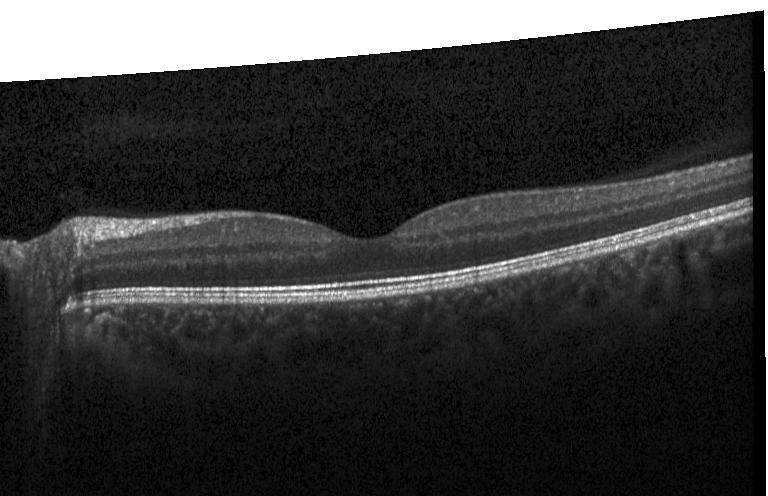 Fovea-centered, optical coherence tomography scan
Finding: no evidence of choroidal neovascularization, diabetic macular edema, or drusen.